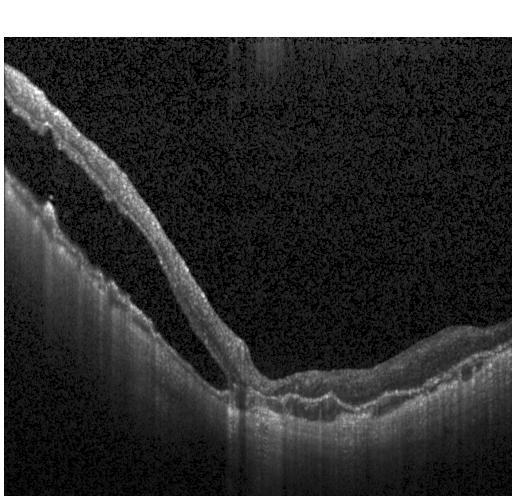

OCT B-scan · macular scan
Finding: a choroidal neovascular membrane.